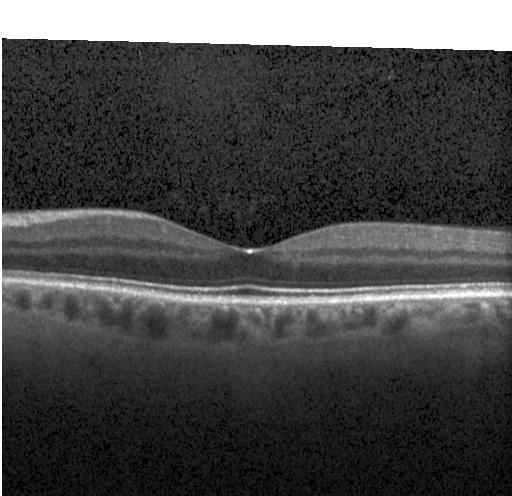 Retinal OCT cross-section showing no evidence of CNV, DME, or drusen.